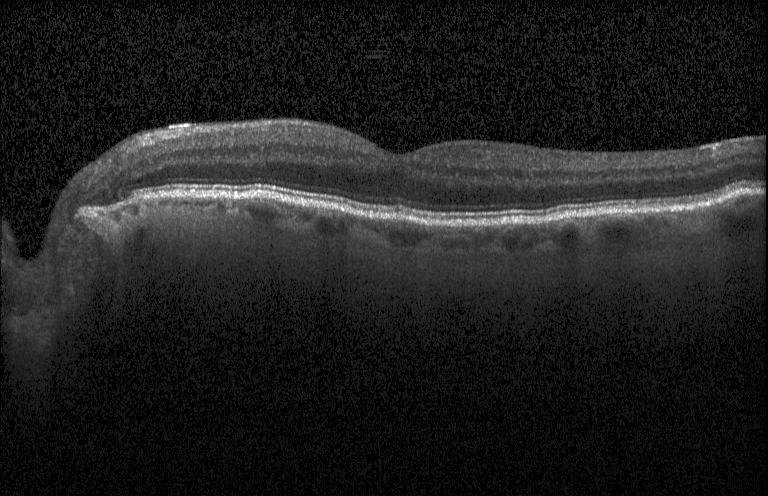

Retinal OCT B-scan. OCT finding: no choroidal neovascularization, no diabetic macular edema, and no drusen.